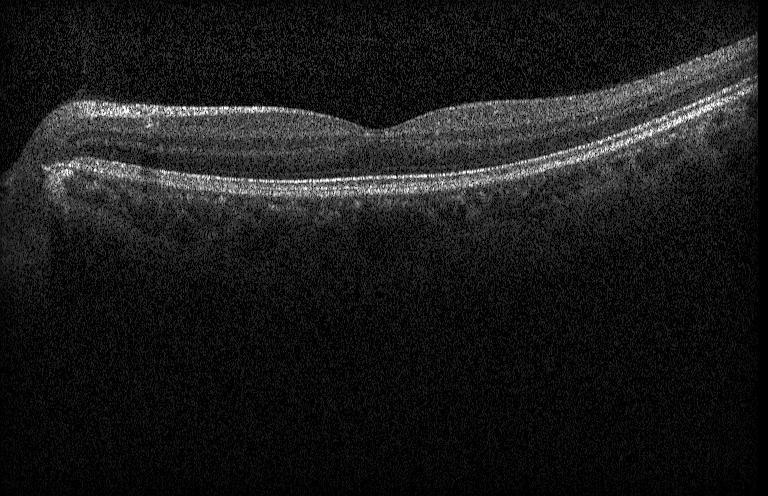
Diagnosis: neither choroidal neovascularization, diabetic macular edema, nor drusen.